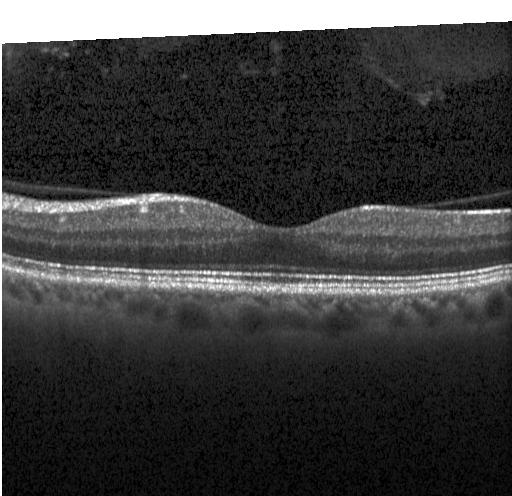

Diagnosis: no choroidal neovascularization, diabetic macular edema, or drusen.